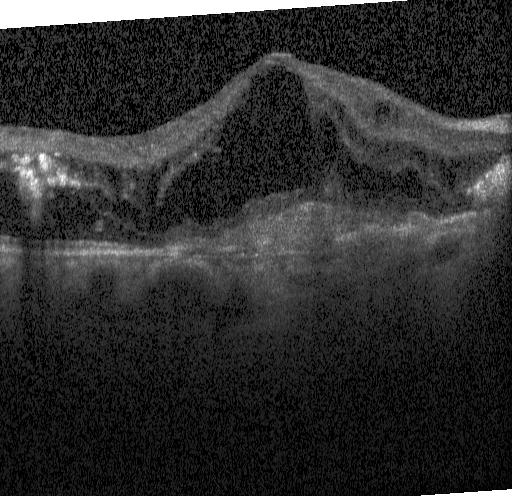
Optical coherence tomography B-scan — The scan shows a choroidal neovascular membrane.